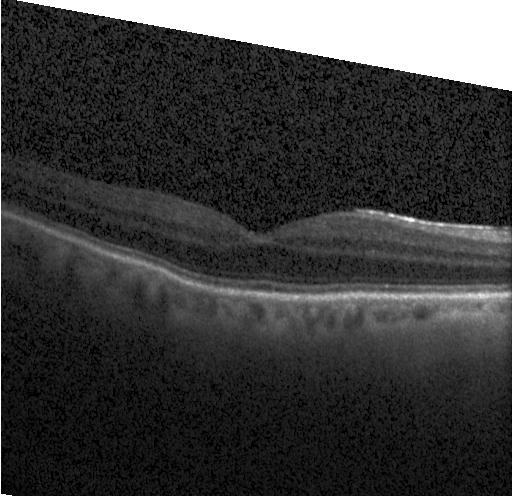 Optical coherence tomography B-scan; acquired on a Heidelberg Spectralis. Assessment: no choroidal neovascularization, no diabetic macular edema, and no drusen.